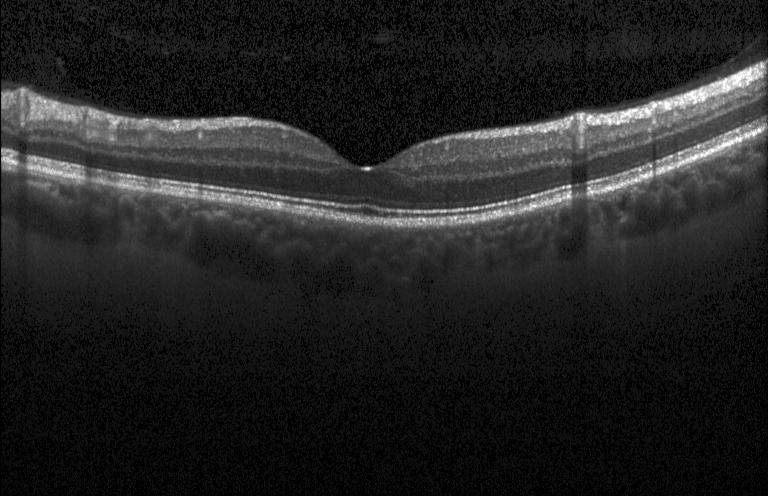

OCT line scan, fovea-centered, instrument: Heidelberg Spectralis.
The scan shows no CNV, no DME, and no drusen.